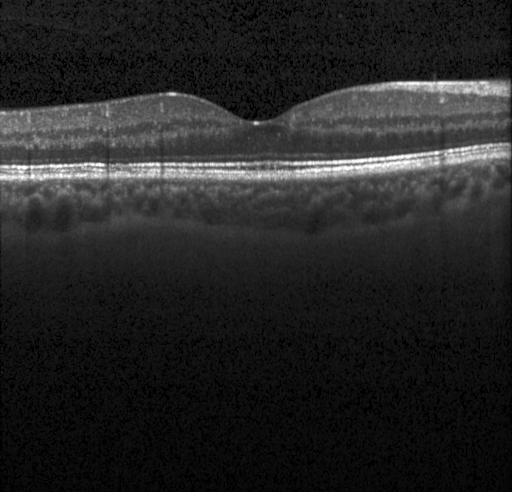 Optical coherence tomography scan. Finding: no choroidal neovascularization, diabetic macular edema, or drusen.